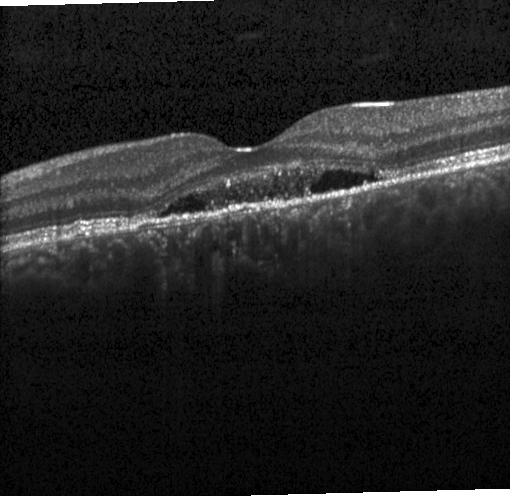
Acquired on a Heidelberg Spectralis · retinal OCT cross-section · macular scan · SD-OCT — This B-scan demonstrates a choroidal neovascular membrane.